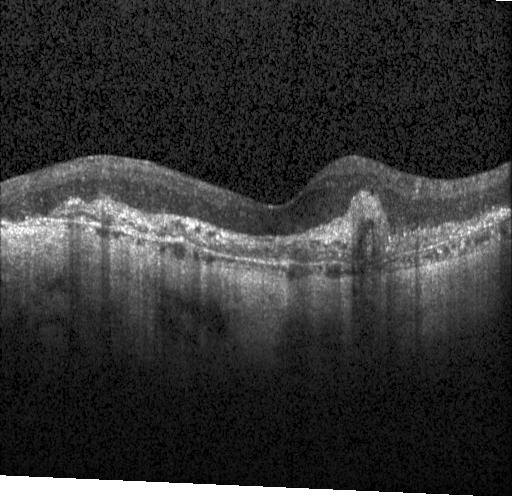
Assessment: a choroidal neovascular membrane.